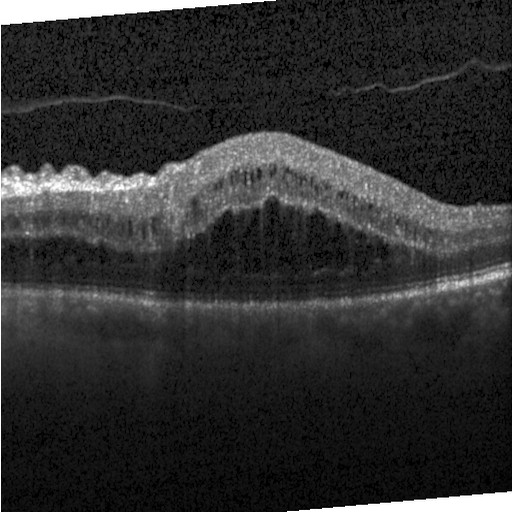
OCT B-scan showing diabetic macular edema (DME).